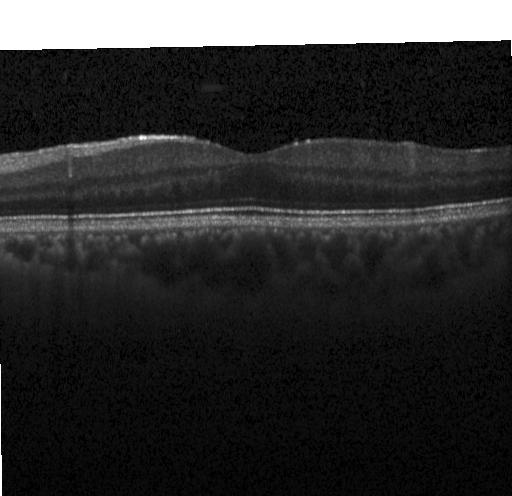

Impression: no evidence of choroidal neovascularization, diabetic macular edema, or drusen.